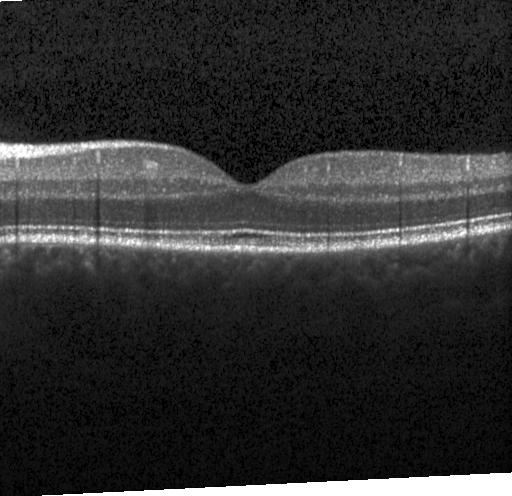
OCT scan showing no evidence of CNV, DME, or drusen.